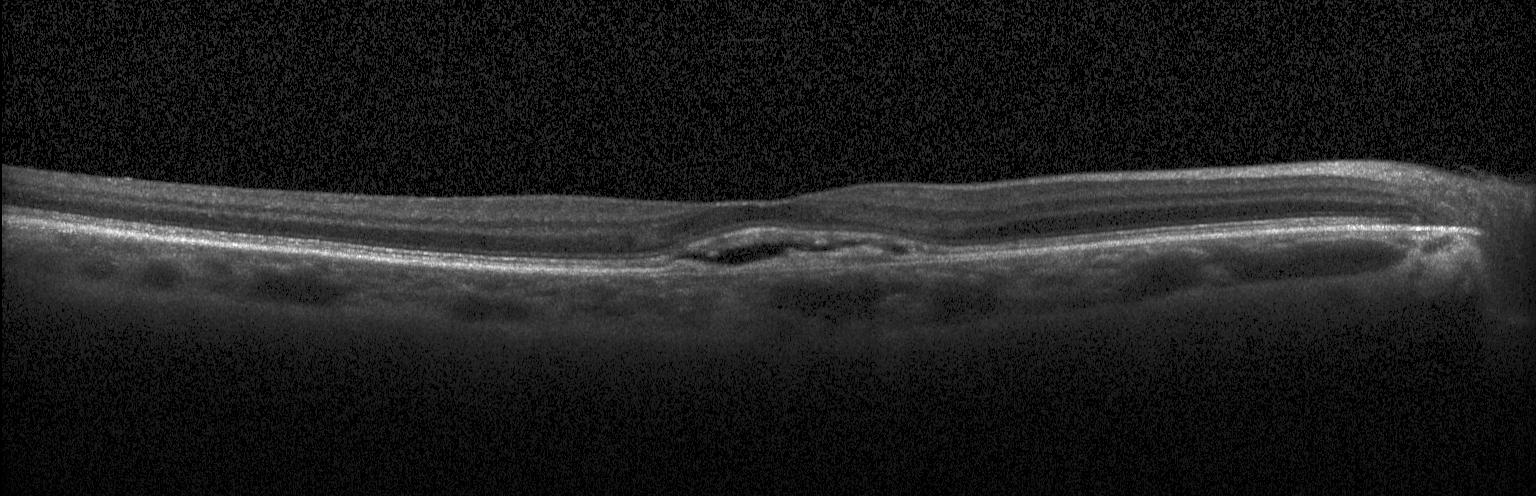
Impression: choroidal neovascularization.